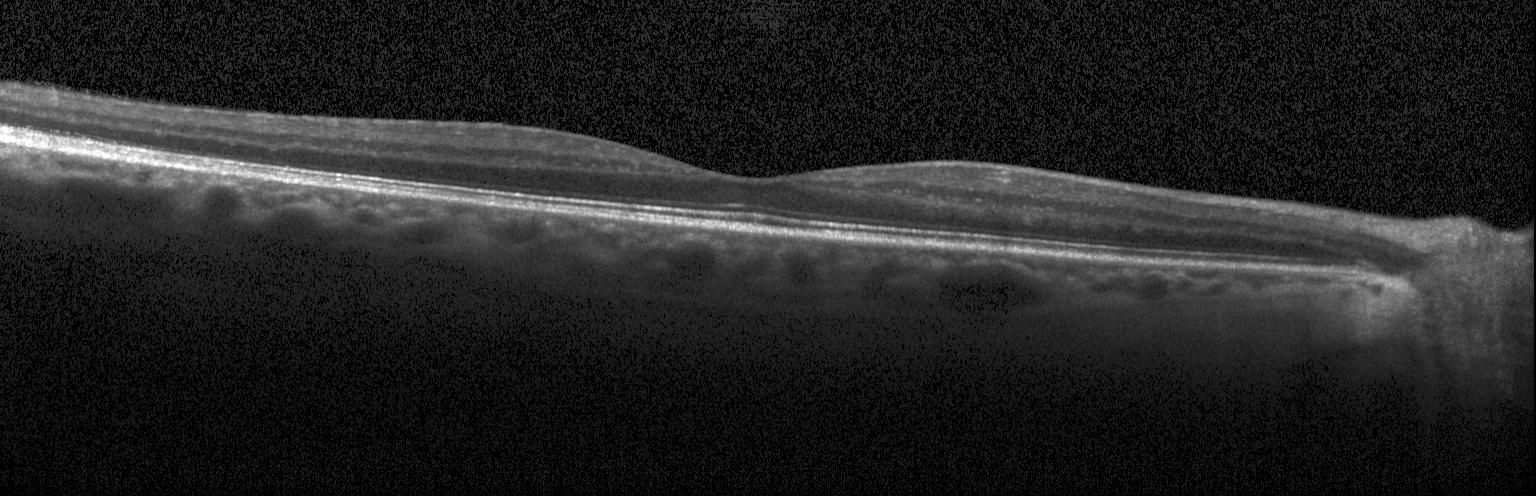
Retinal OCT cross-section · fovea-centered
Impression: no choroidal neovascularization, no diabetic macular edema, and no drusen.